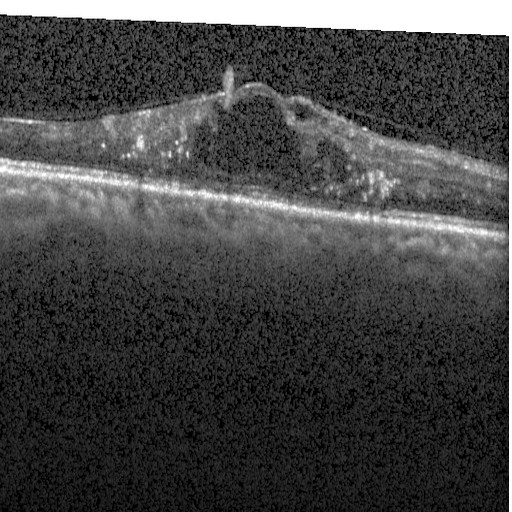 Impression: diabetic macular edema.